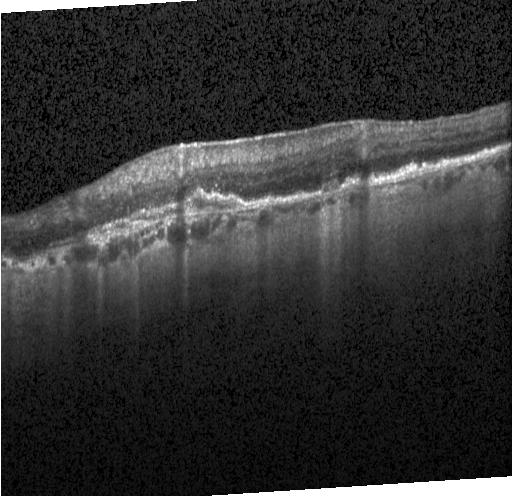 Retinal OCT B-scan.
Finding: a choroidal neovascular membrane.